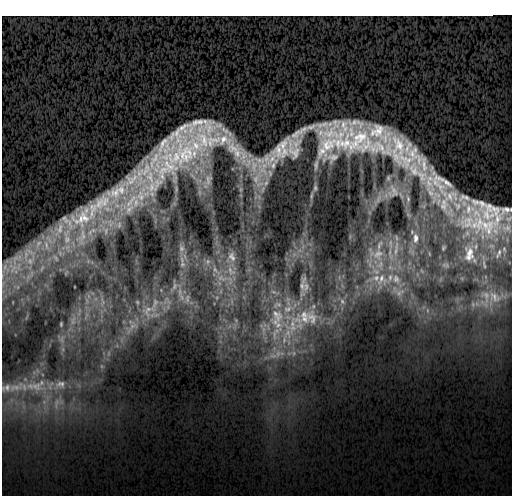 OCT line scan. Heidelberg Spectralis.
This B-scan demonstrates a choroidal neovascular membrane.